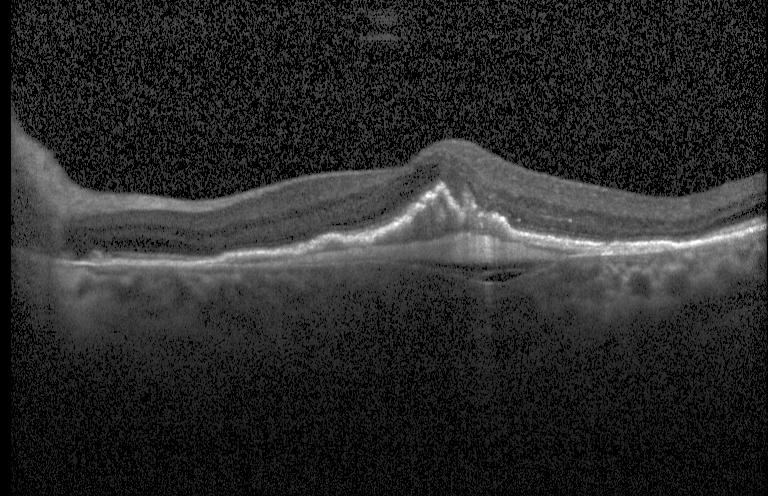

Retinal OCT cross-section; fovea-centered. Macular OCT: a choroidal neovascular membrane.